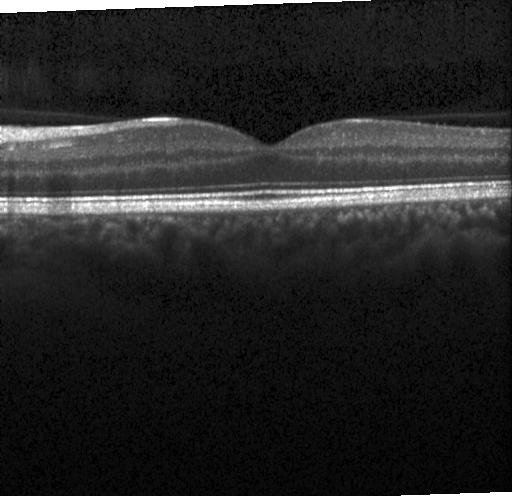

Dx: no choroidal neovascularization, no diabetic macular edema, and no drusen.